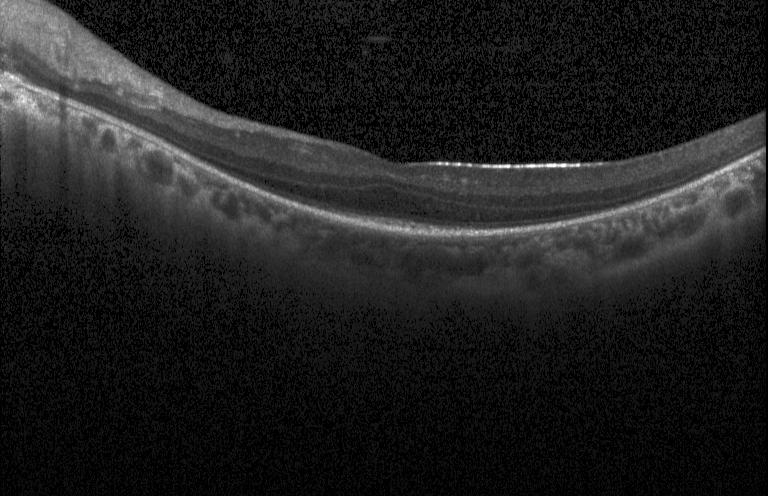
Heidelberg Spectralis · centered on the fovea · retinal OCT cross-section · spectral-domain OCT
Assessment: no CNV, no DME, and no drusen.